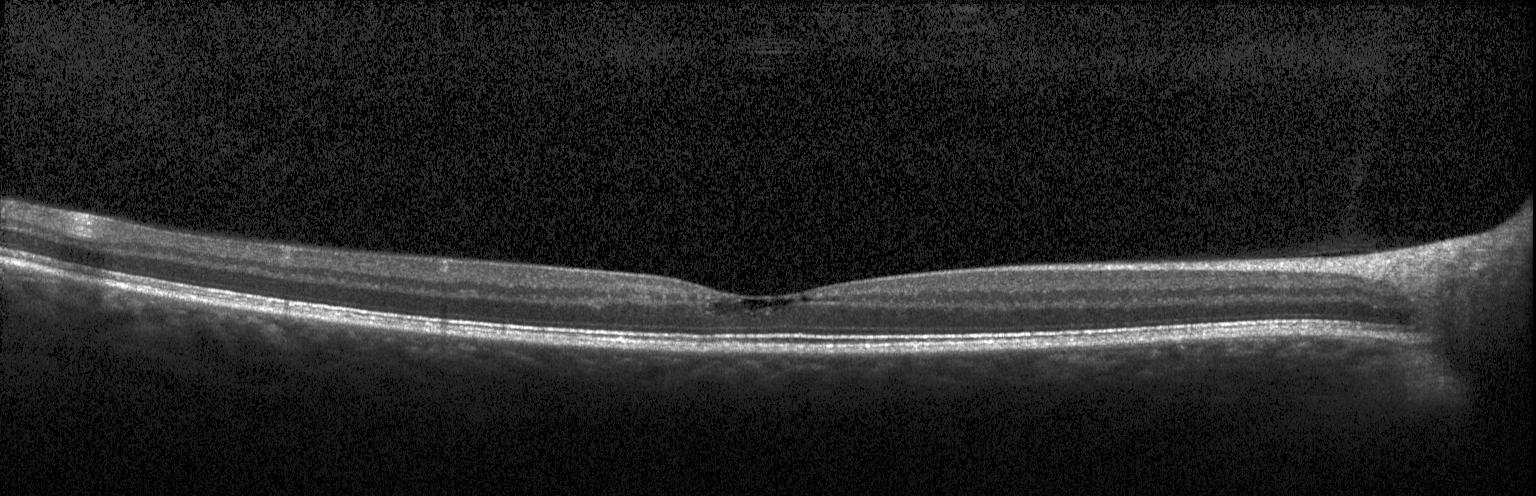
Heidelberg Spectralis OCT system, horizontal scan through the fovea, optical coherence tomography scan
The scan shows diabetic macular edema.